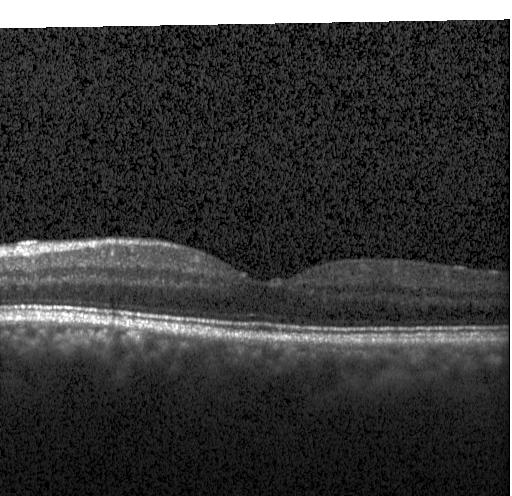 Retinal OCT B-scan. The scan shows neither CNV, DME, nor drusen.